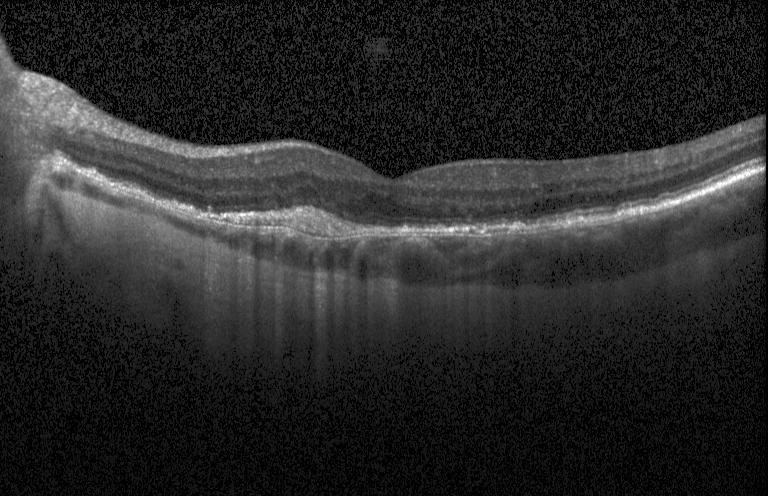

Dx: a choroidal neovascular membrane.